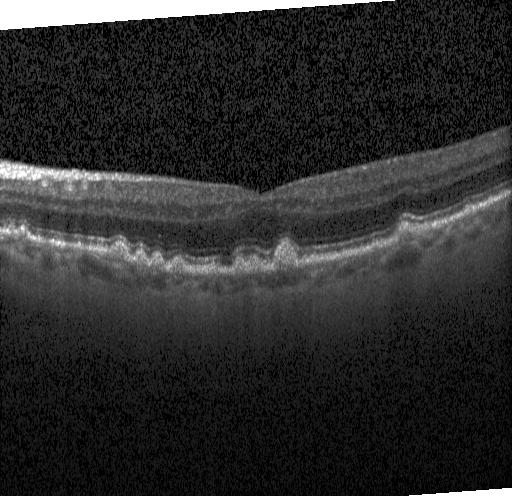

Diagnosis: multiple drusen.